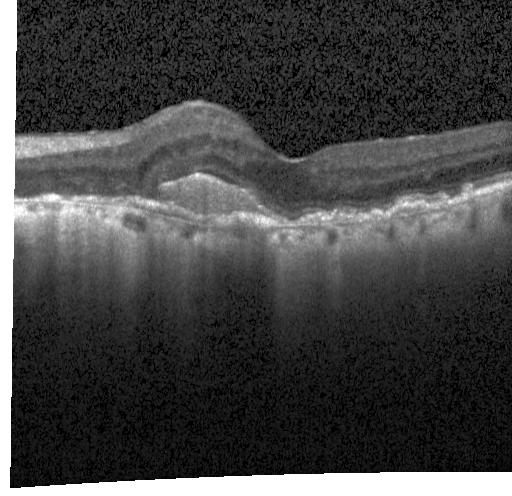
The scan shows a choroidal neovascular membrane.